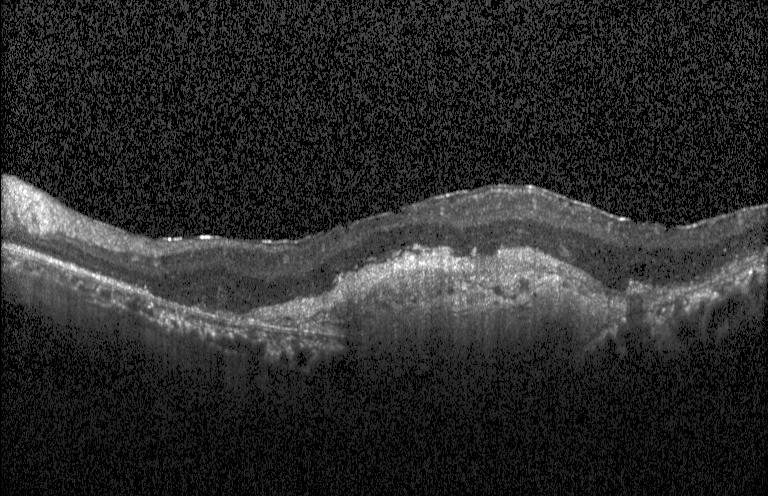 A choroidal neovascular membrane.